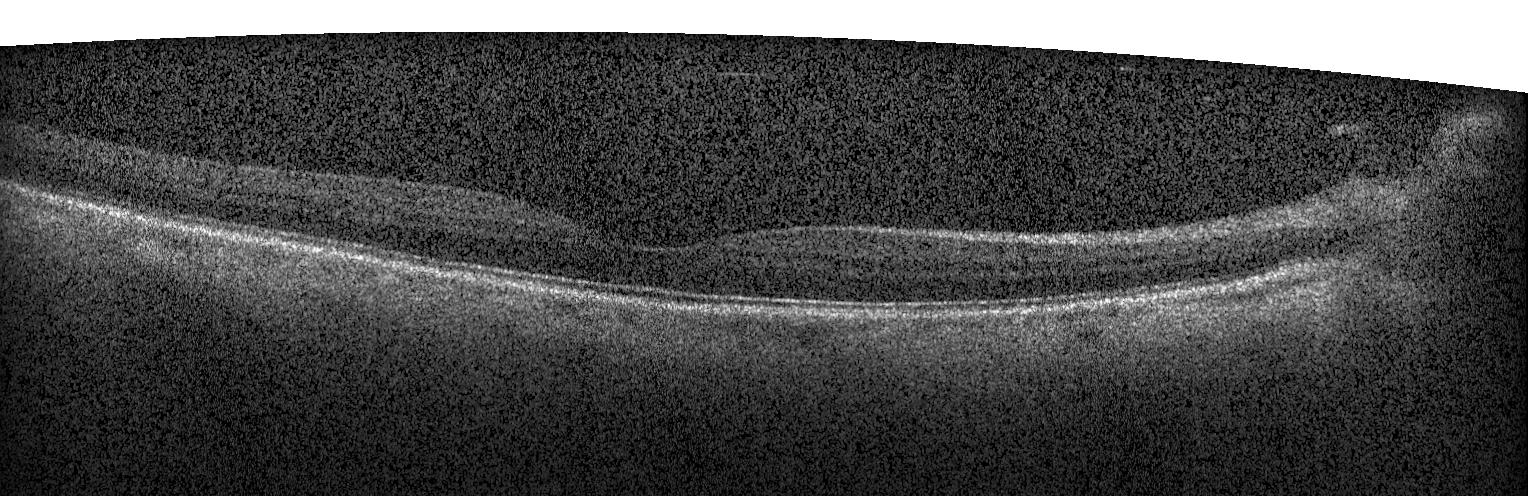

Heidelberg Spectralis; retinal OCT cross-section; spectral-domain optical coherence tomography. Impression: no CNV, DME, or drusen.